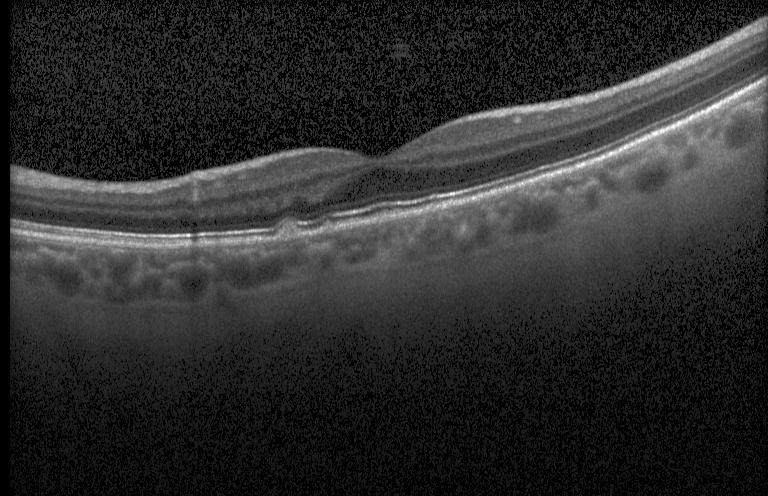
Retinal OCT B-scan
Diagnosis: multiple drusen.